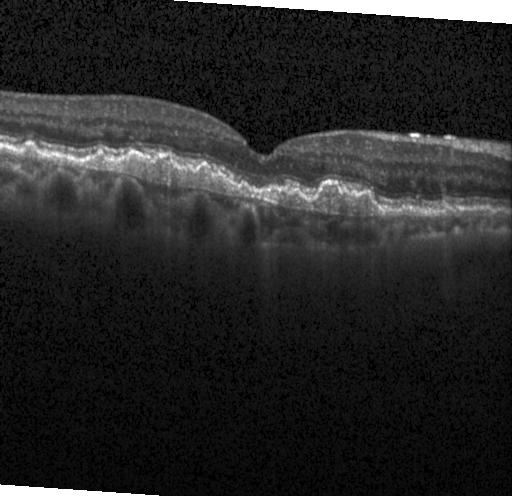

Spectral-domain OCT. Instrument: Heidelberg Spectralis. Retinal OCT B-scan — Assessment: a choroidal neovascular membrane.